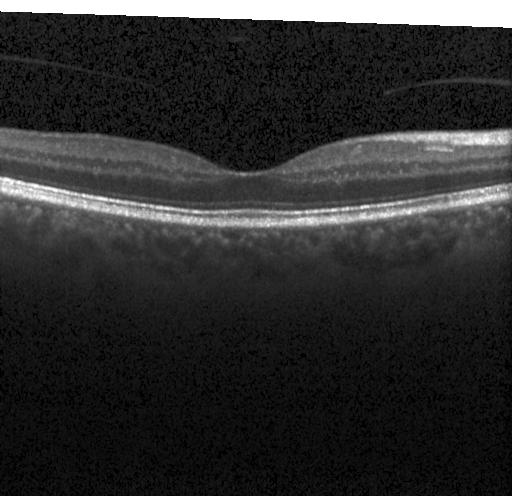
OCT B-scan
Diagnosis: no CNV, no DME, and no drusen.